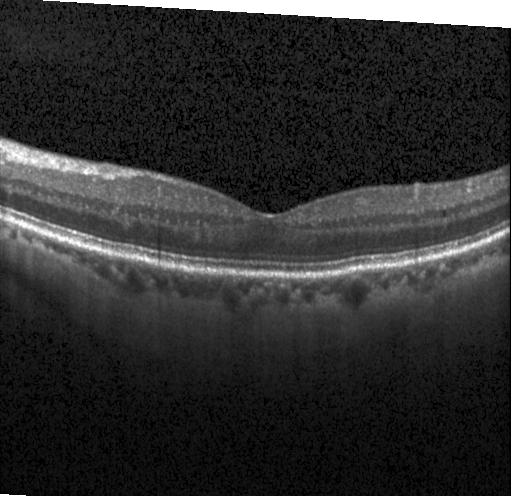
Retinal OCT cross-section showing no choroidal neovascularization, diabetic macular edema, or drusen.